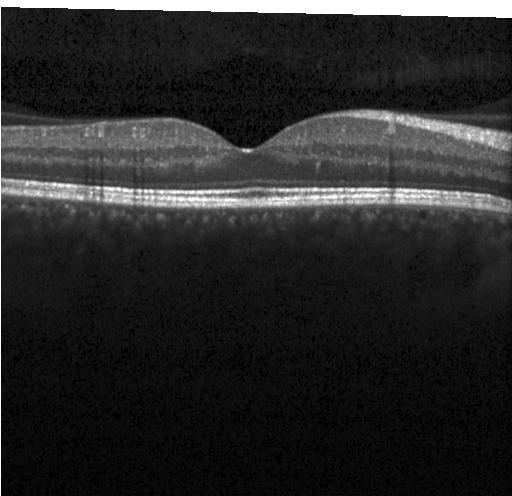 Spectral-domain OCT. OCT line scan
Assessment: no choroidal neovascularization, no diabetic macular edema, and no drusen.